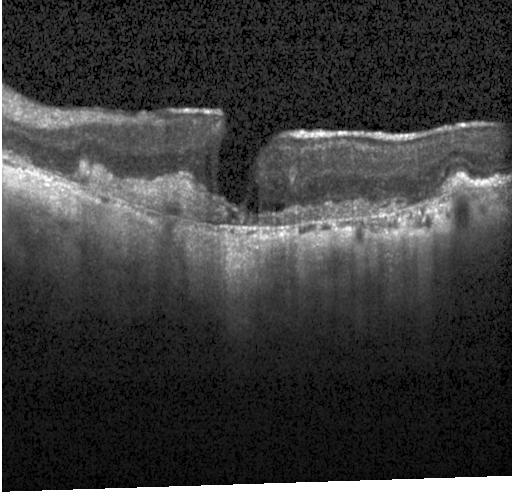 Heidelberg Spectralis; OCT line scan
Macular OCT: choroidal neovascularization.